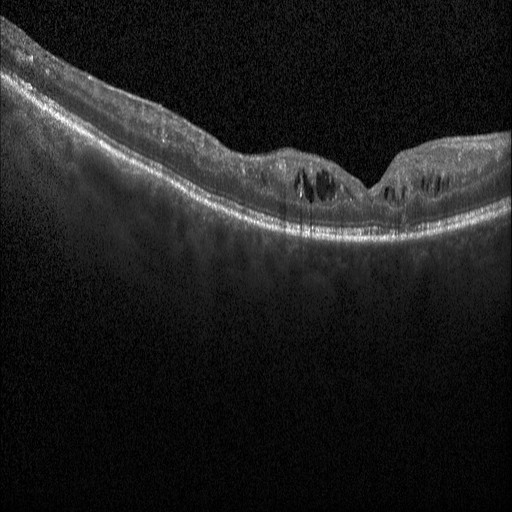 Optical coherence tomography B-scan · spectral-domain OCT — Macular OCT: DME.